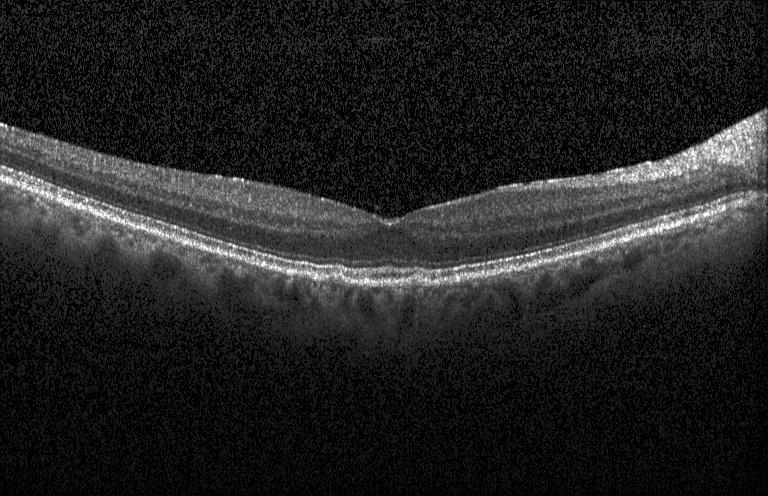
Impression: drusen.